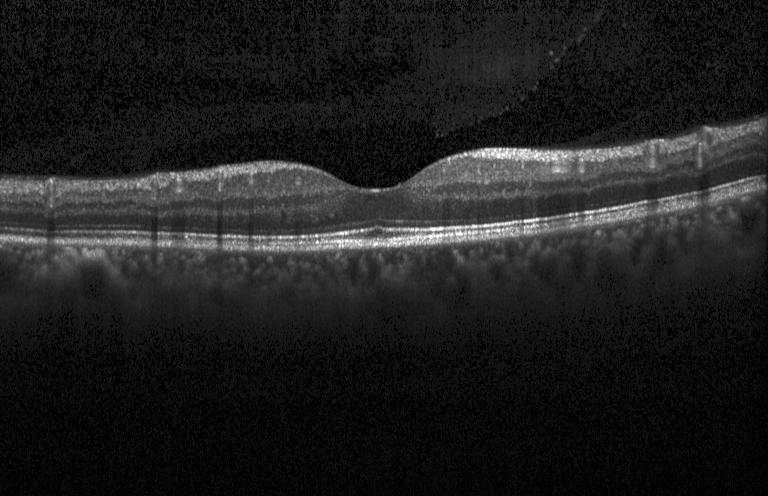
Spectral-domain optical coherence tomography; centered on the fovea; Heidelberg Spectralis OCT system; optical coherence tomography B-scan — Macular OCT: no choroidal neovascularization, diabetic macular edema, or drusen.